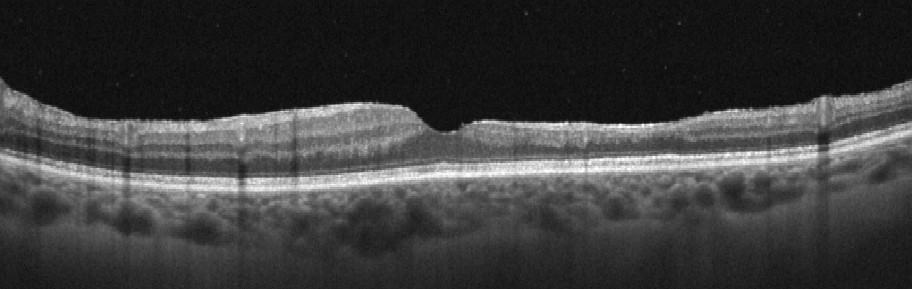 Macular scan. OCT line scan
Finding: RVO.